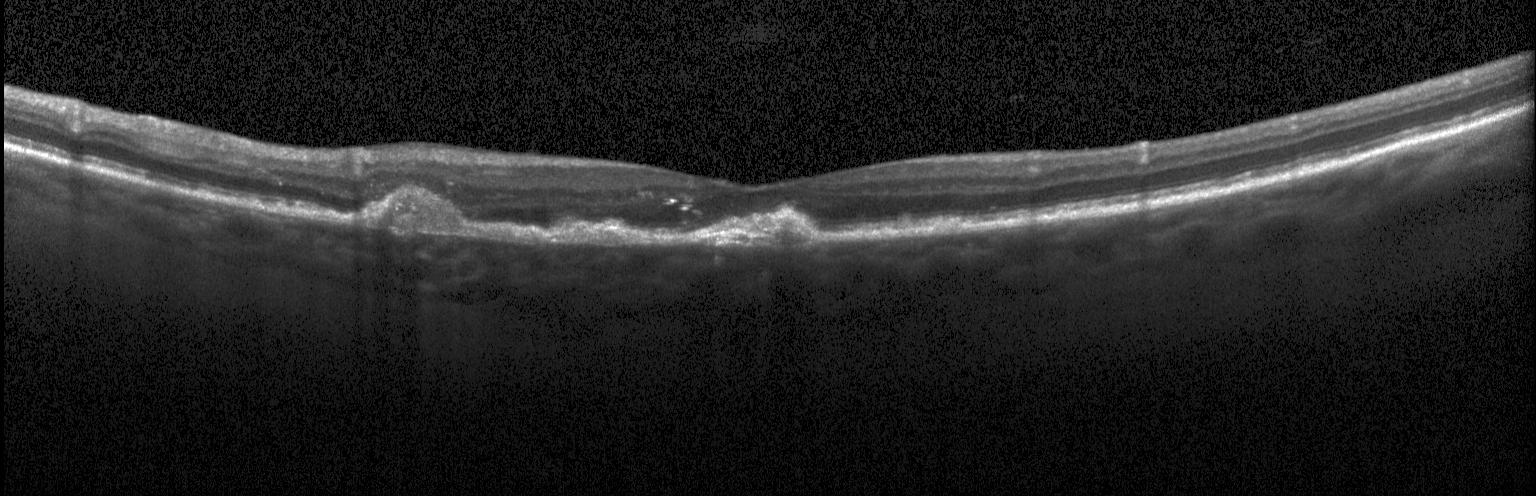
Diagnosis: a choroidal neovascular membrane.